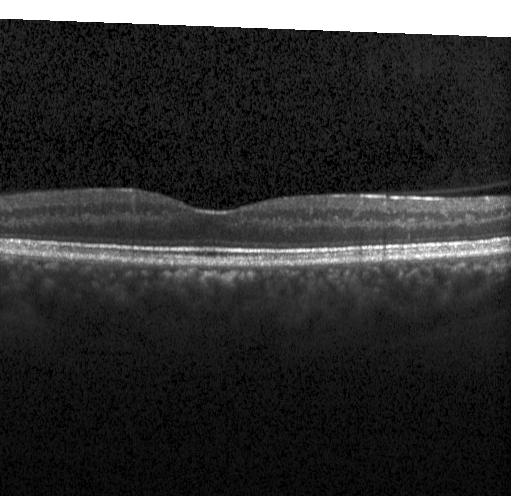
Impression: neither choroidal neovascularization, diabetic macular edema, nor drusen.